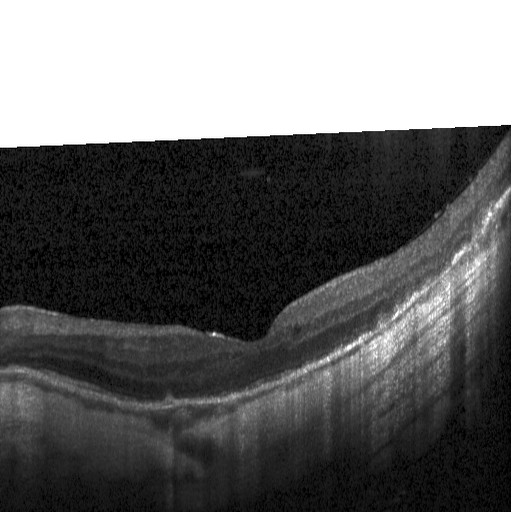 Optical coherence tomography B-scan. Spectral-domain optical coherence tomography — Assessment: diabetic macular edema (DME).